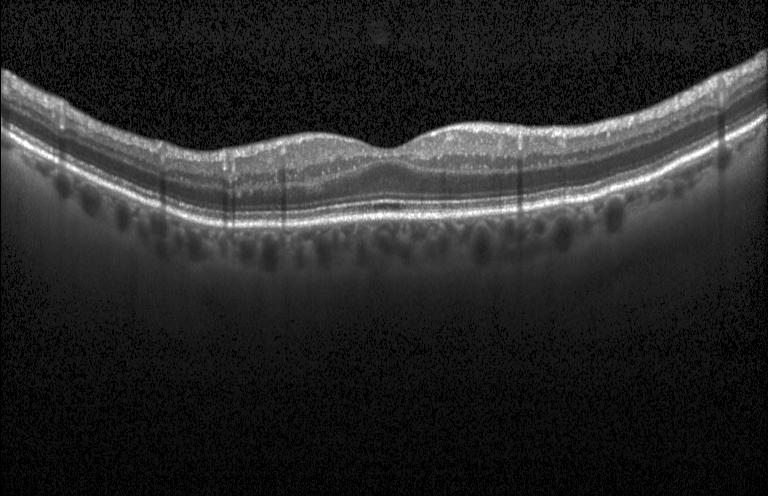
Retinal OCT cross-section showing no choroidal neovascularization, no diabetic macular edema, and no drusen.